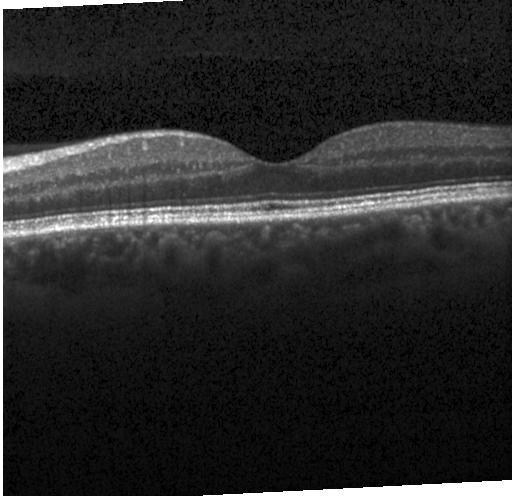

Diagnosis: no CNV, no DME, and no drusen.